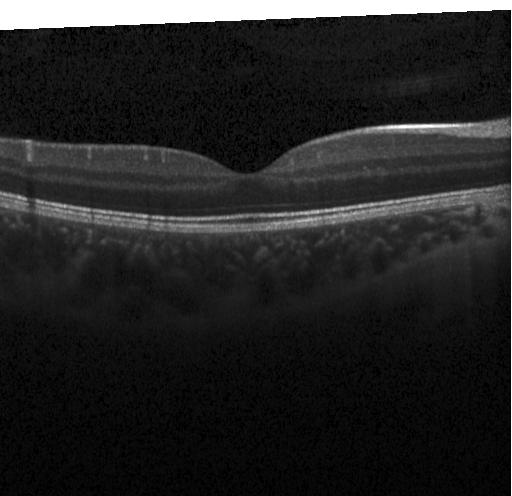 Finding: neither choroidal neovascularization, diabetic macular edema, nor drusen.